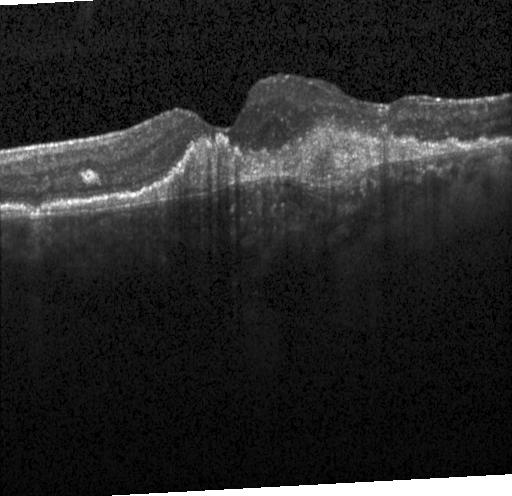
Retinal OCT cross-section; spectral-domain optical coherence tomography
Dx: a choroidal neovascular membrane.